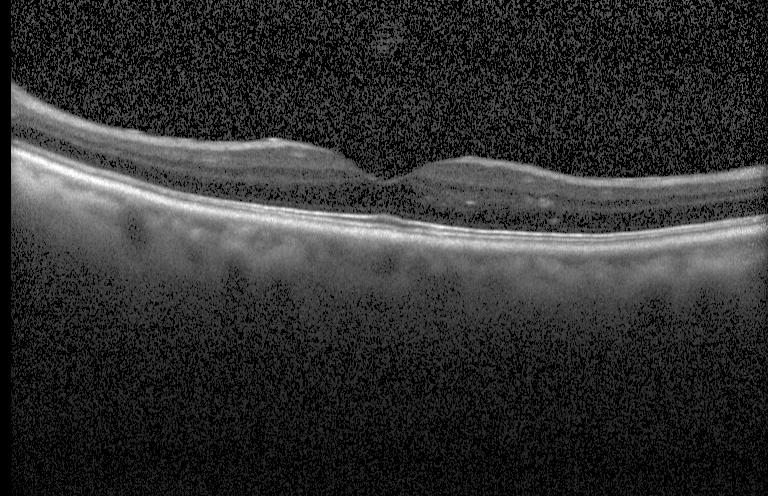 OCT finding: no choroidal neovascularization, diabetic macular edema, or drusen.